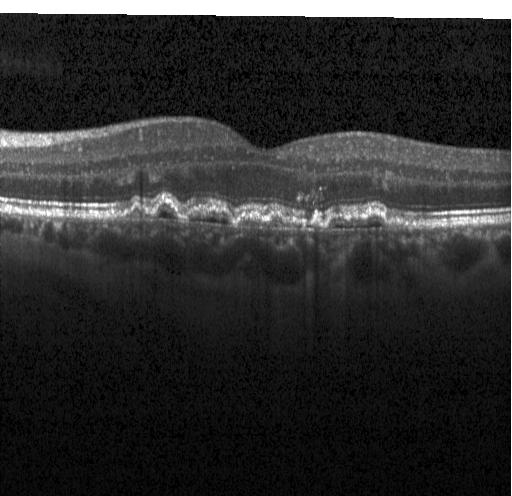

Retinal OCT B-scan, centered on the fovea, spectral-domain optical coherence tomography
Finding: drusen.